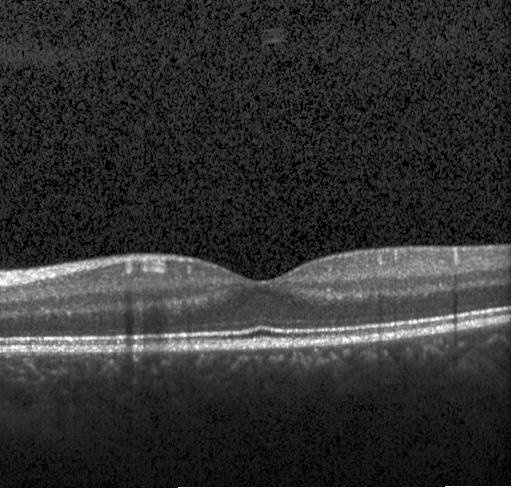

OCT finding: no choroidal neovascularization, diabetic macular edema, or drusen.